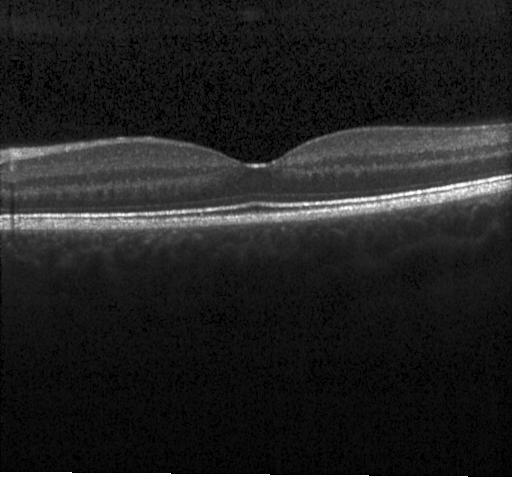

Macular OCT: no evidence of choroidal neovascularization, diabetic macular edema, or drusen.